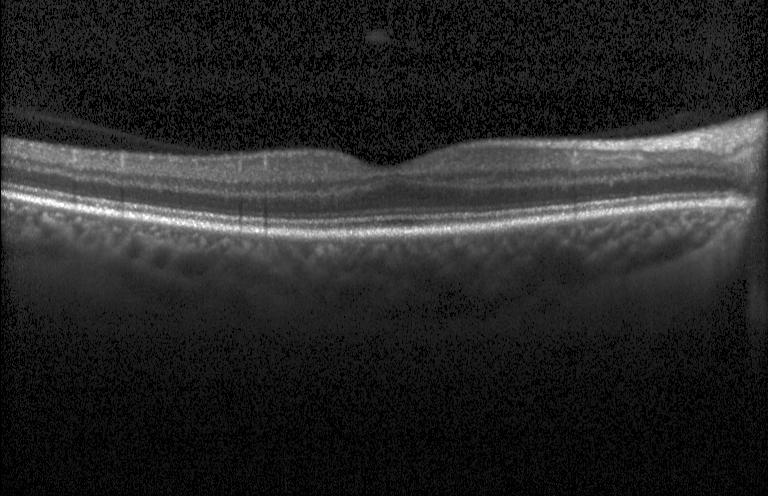

Retinal OCT cross-section · acquired on a Heidelberg Spectralis. Dx: no CNV, no DME, and no drusen.